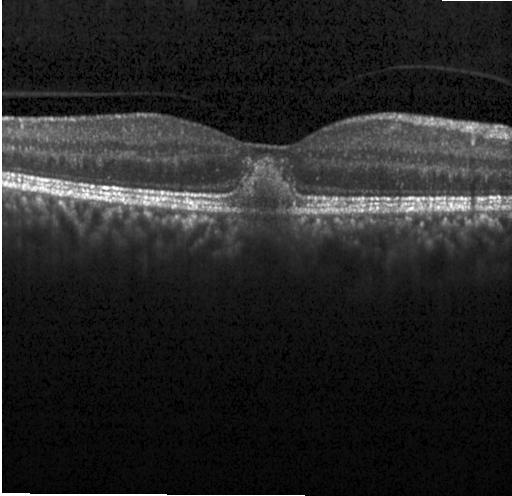 OCT finding: a choroidal neovascular membrane.